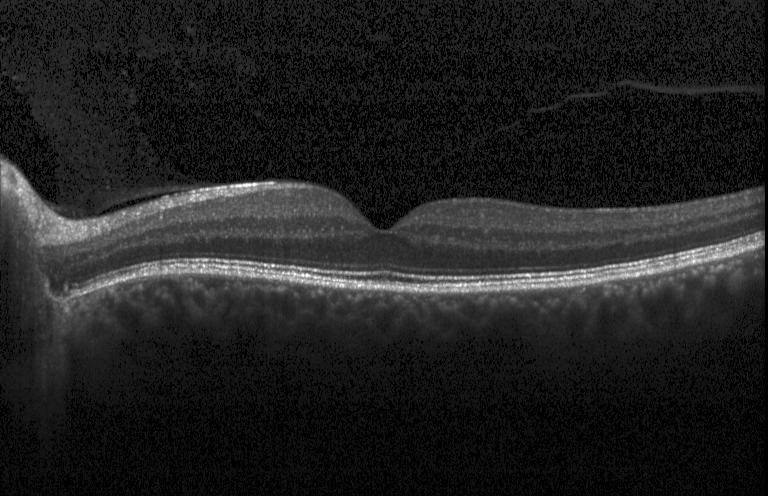
OCT B-scan showing neither choroidal neovascularization, diabetic macular edema, nor drusen.